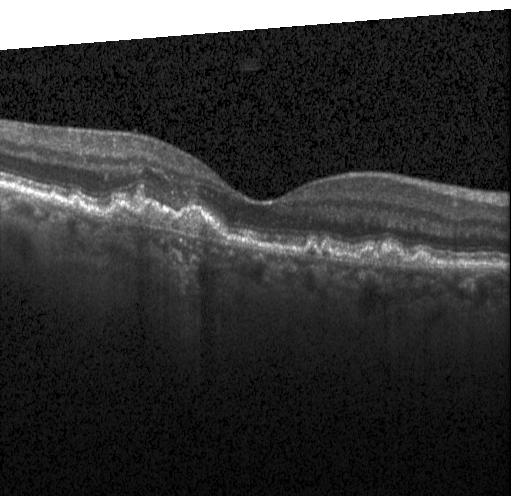 Spectral-domain OCT B-scan: a choroidal neovascular membrane.